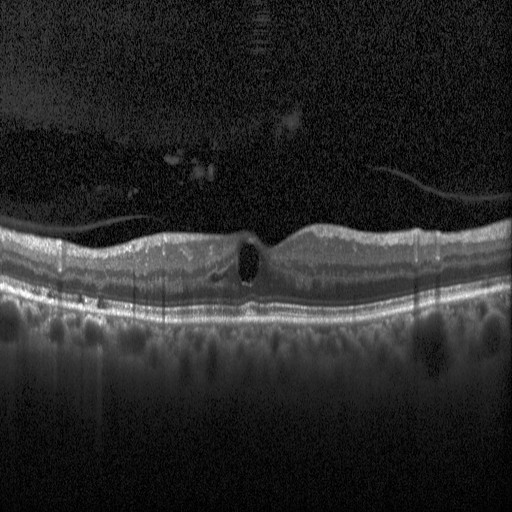 Fovea-centered, retinal OCT B-scan, spectral-domain OCT, Heidelberg Spectralis OCT system
This B-scan demonstrates diabetic macular edema (DME).